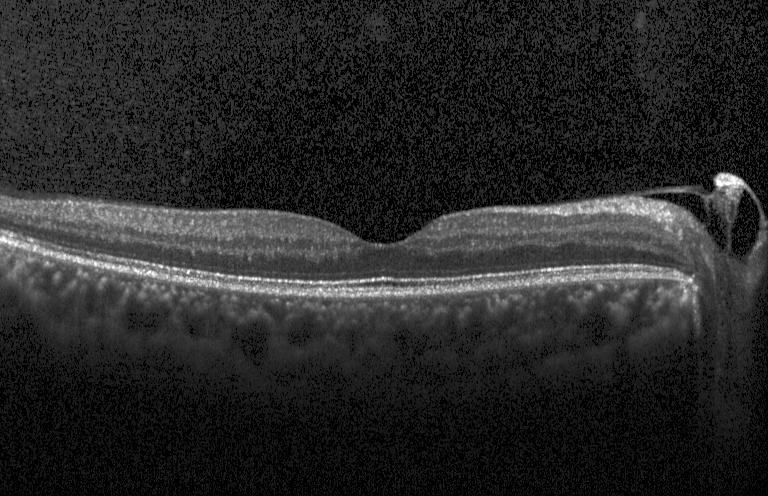

Retinal OCT B-scan — The scan shows no choroidal neovascularization, no diabetic macular edema, and no drusen.